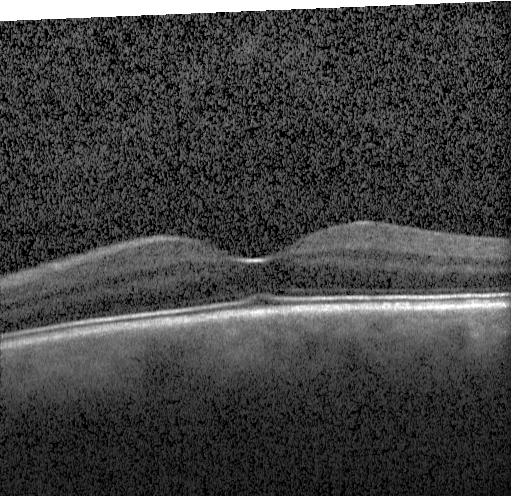

Fovea-centered. Heidelberg Spectralis OCT system. Retinal OCT B-scan. SD-OCT — Diagnosis: no choroidal neovascularization, no diabetic macular edema, and no drusen.